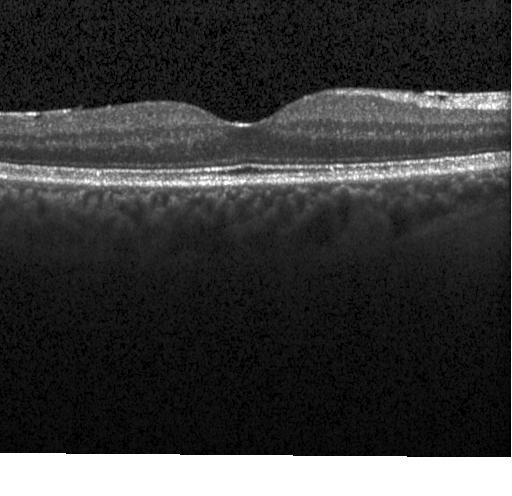

Through the macula, instrument: Heidelberg Spectralis, OCT B-scan
Diagnosis: no evidence of choroidal neovascularization, diabetic macular edema, or drusen.